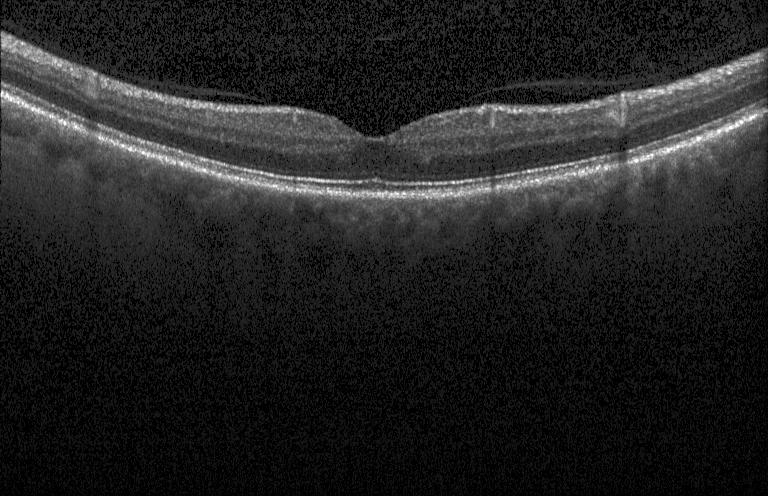
Instrument: Heidelberg Spectralis, through the macula, optical coherence tomography B-scan.
No choroidal neovascularization, diabetic macular edema, or drusen.